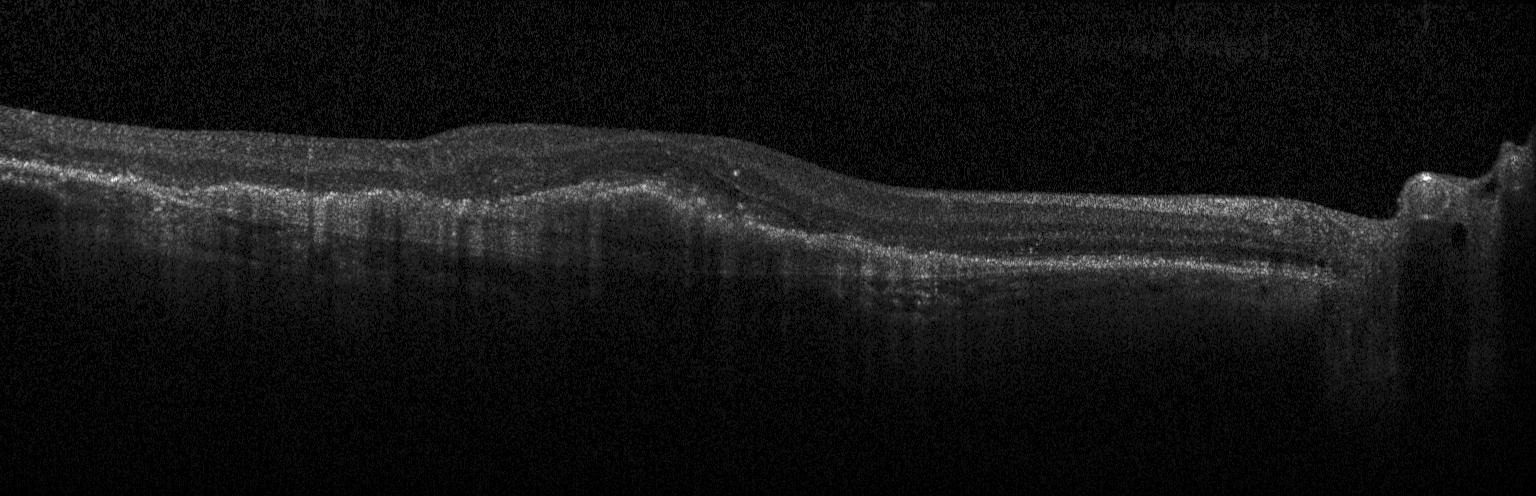
Centered on the fovea; retinal OCT B-scan — Impression: choroidal neovascularization.